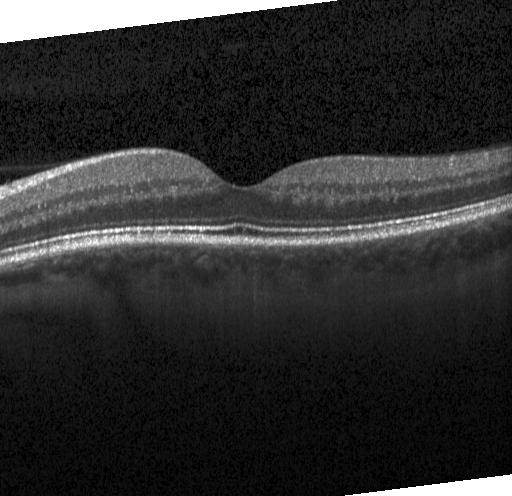

Optical coherence tomography B-scan — Impression: no evidence of choroidal neovascularization, diabetic macular edema, or drusen.